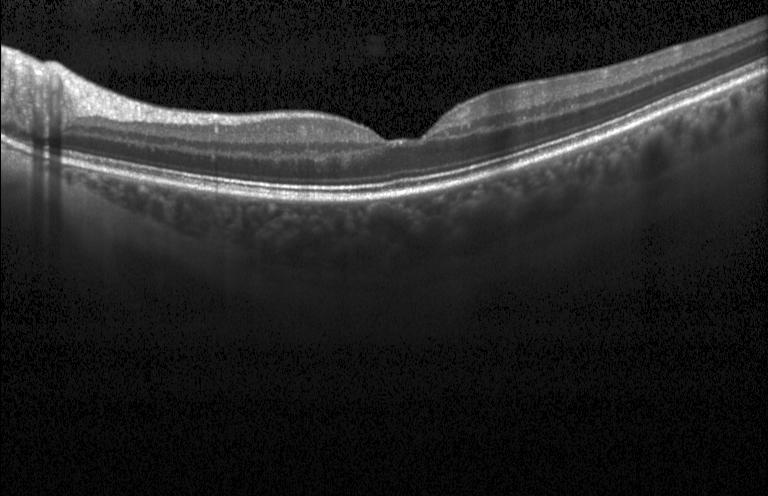 Dx: no choroidal neovascularization, diabetic macular edema, or drusen.